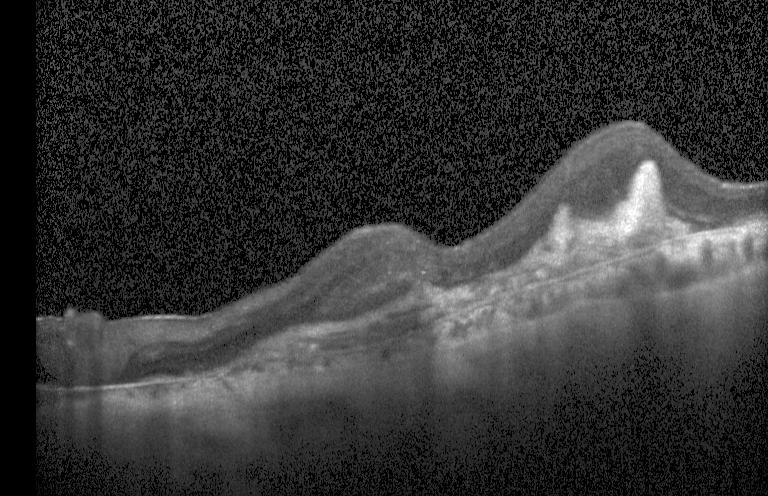
This B-scan demonstrates a choroidal neovascular membrane.